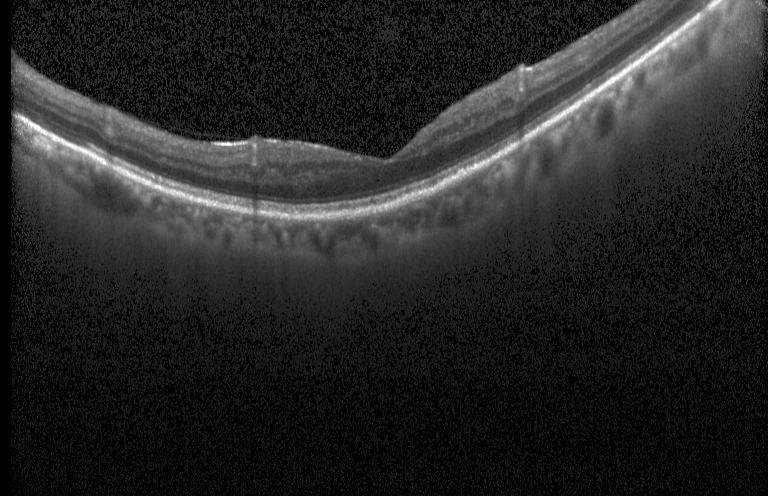 OCT line scan, macular scan, spectral-domain optical coherence tomography, Heidelberg Spectralis
Impression: neither choroidal neovascularization, diabetic macular edema, nor drusen.